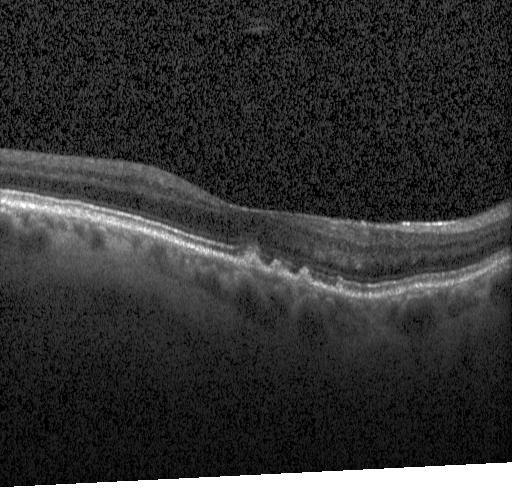 Diagnosis: drusen.